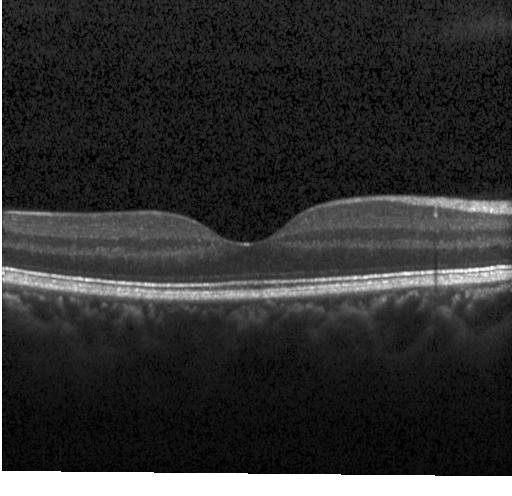 Through the macula; optical coherence tomography scan; Heidelberg Spectralis OCT system; SD-OCT.
Macular OCT: no evidence of choroidal neovascularization, diabetic macular edema, or drusen.